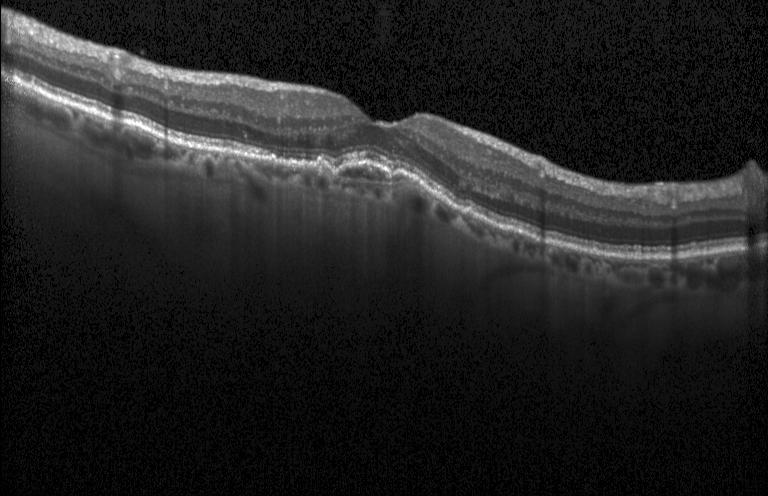

OCT B-scan showing a choroidal neovascular membrane.